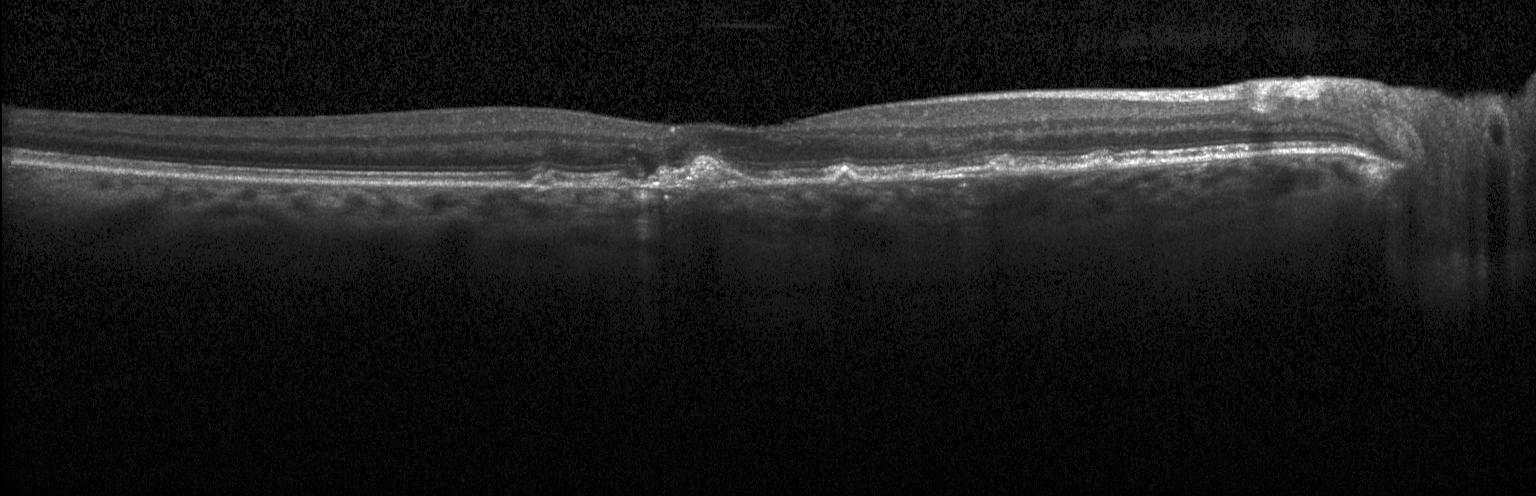 Macular OCT: choroidal neovascularization.